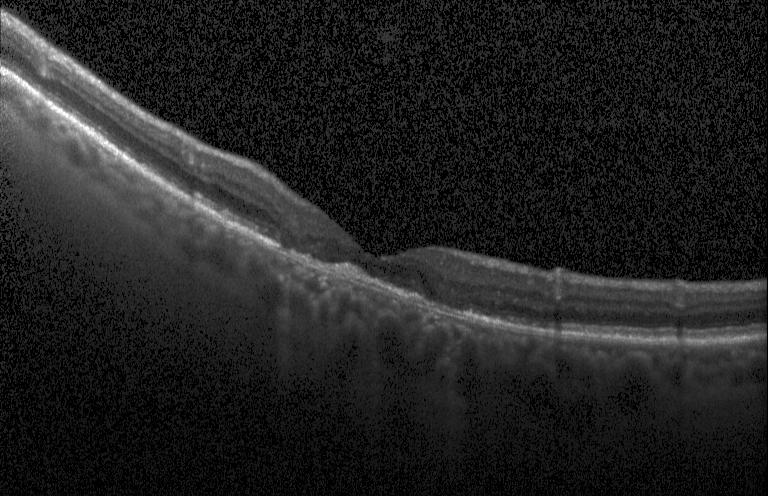

The scan shows a choroidal neovascular membrane.